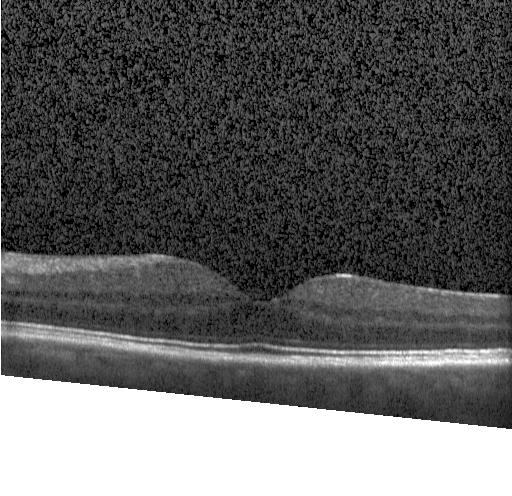
Macular scan, OCT line scan, Heidelberg Spectralis OCT system, SD-OCT. Diagnosis: no choroidal neovascularization, diabetic macular edema, or drusen.